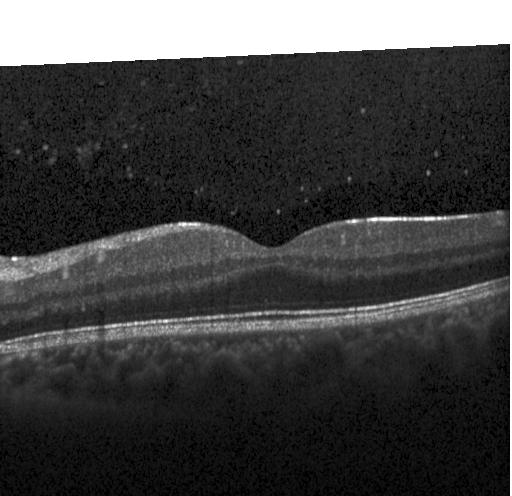

Finding: neither choroidal neovascularization, diabetic macular edema, nor drusen.